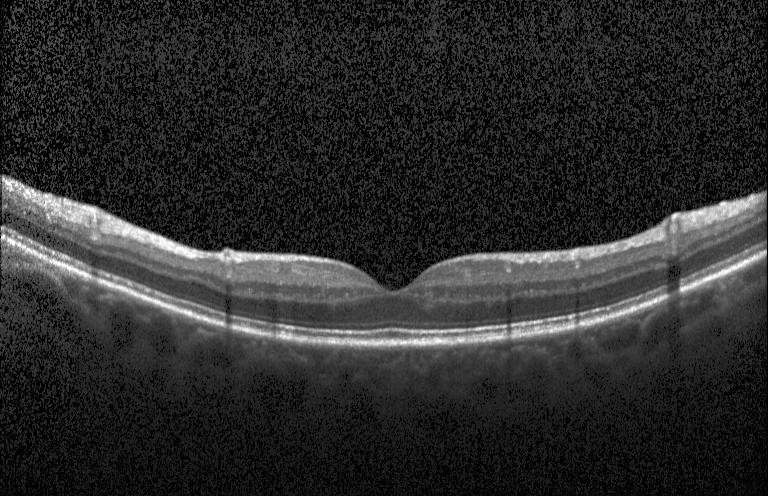

Impression: neither CNV, DME, nor drusen.